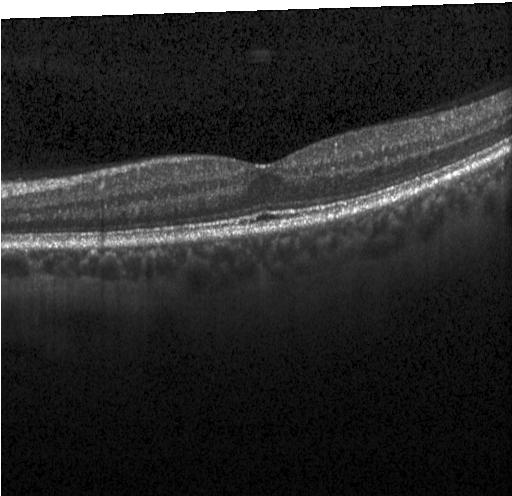 Retinal OCT B-scan; instrument: Heidelberg Spectralis
The scan shows neither CNV, DME, nor drusen.